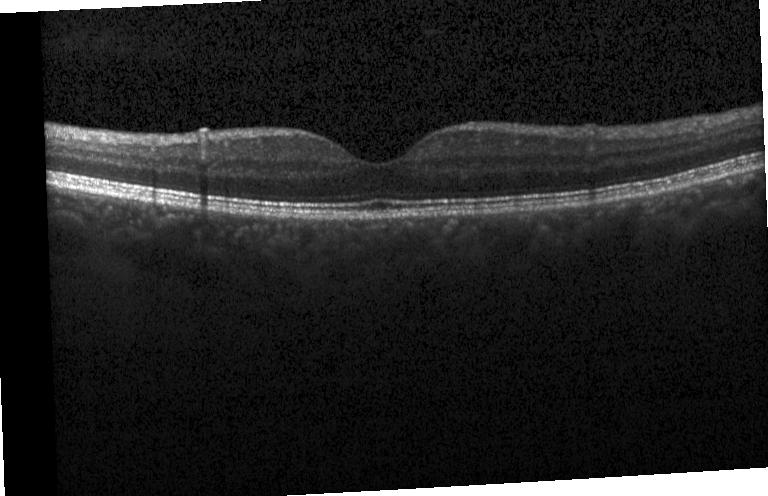

Acquired on a Heidelberg Spectralis, horizontal scan through the fovea, retinal OCT cross-section
Dx: no choroidal neovascularization, diabetic macular edema, or drusen.